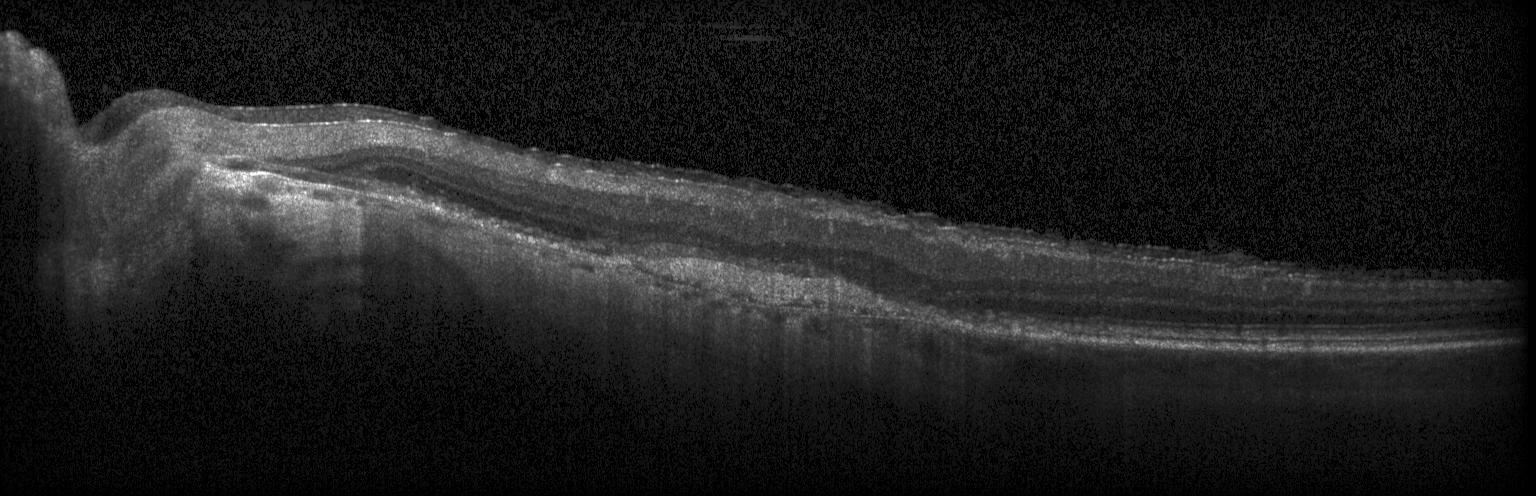 OCT finding: a choroidal neovascular membrane.